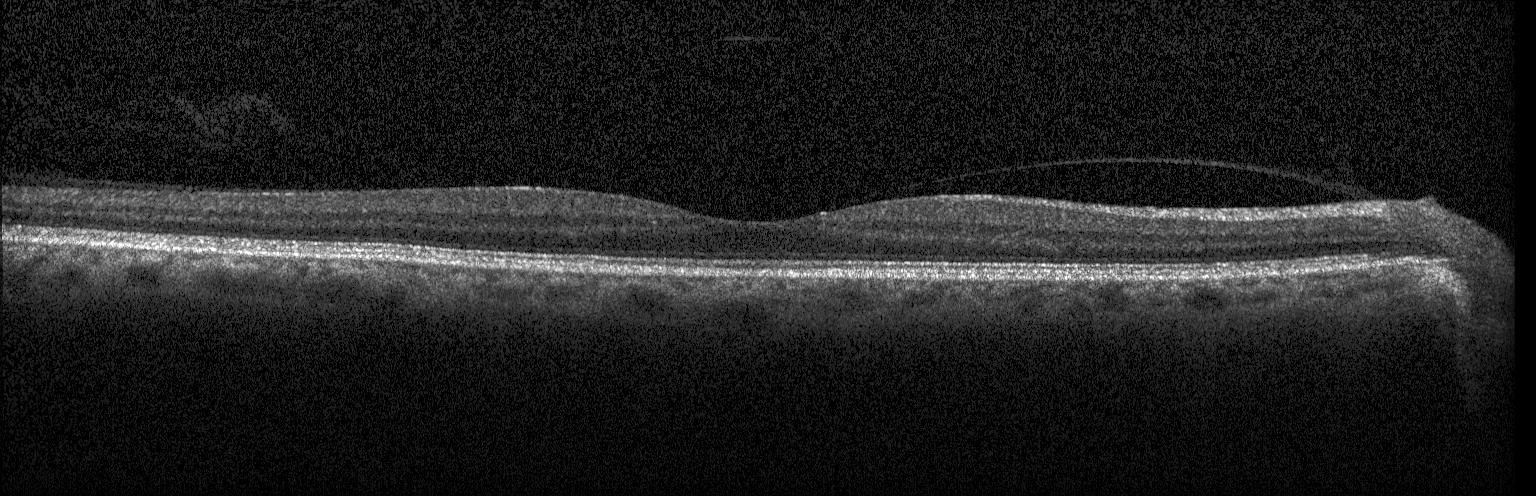

Optical coherence tomography scan. Diagnosis: neither choroidal neovascularization, diabetic macular edema, nor drusen.